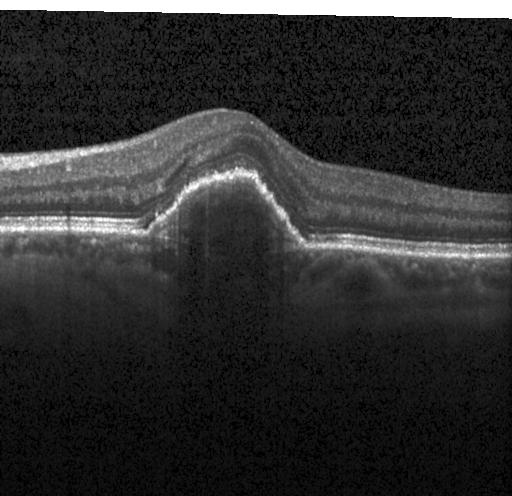

Finding: choroidal neovascularization.